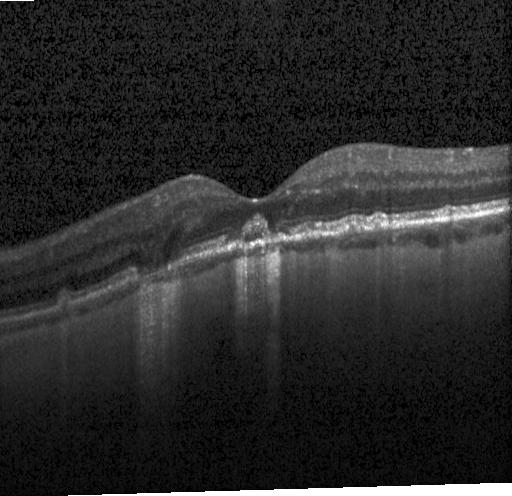

Spectral-domain OCT B-scan: a choroidal neovascular membrane.